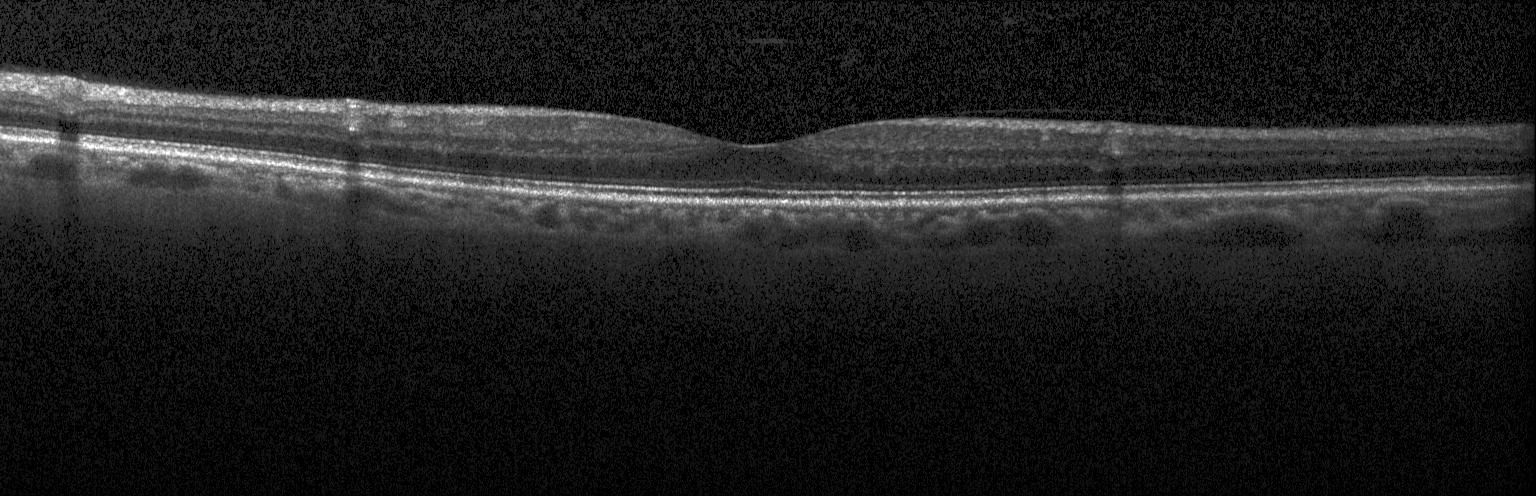
Dx: no choroidal neovascularization, diabetic macular edema, or drusen.